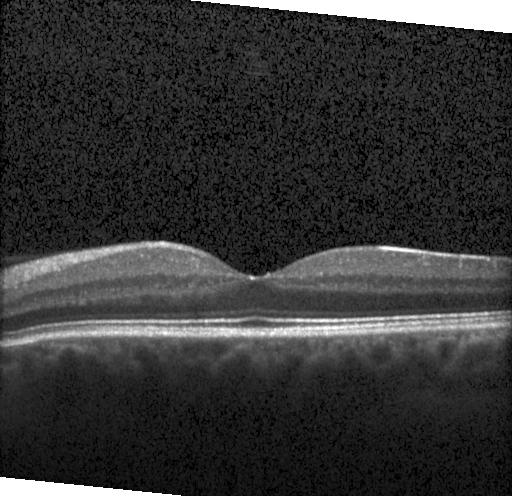

Through the macula; OCT B-scan; Heidelberg Spectralis OCT system; SD-OCT
Dx: neither CNV, DME, nor drusen.